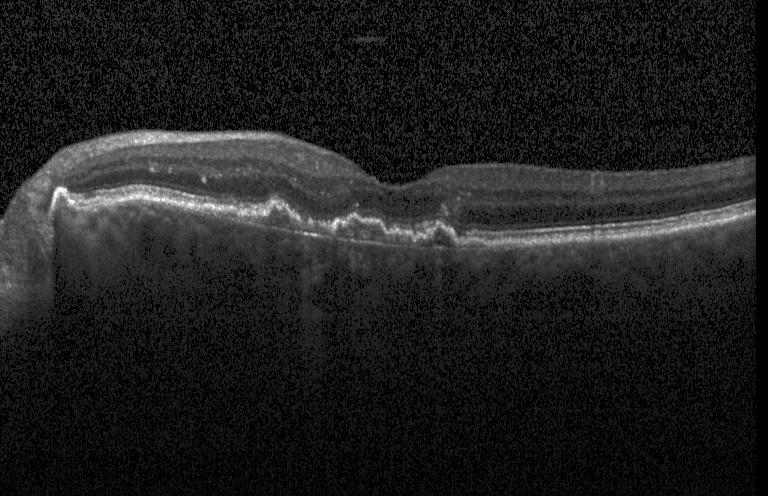
Retinal OCT cross-section — CNV.